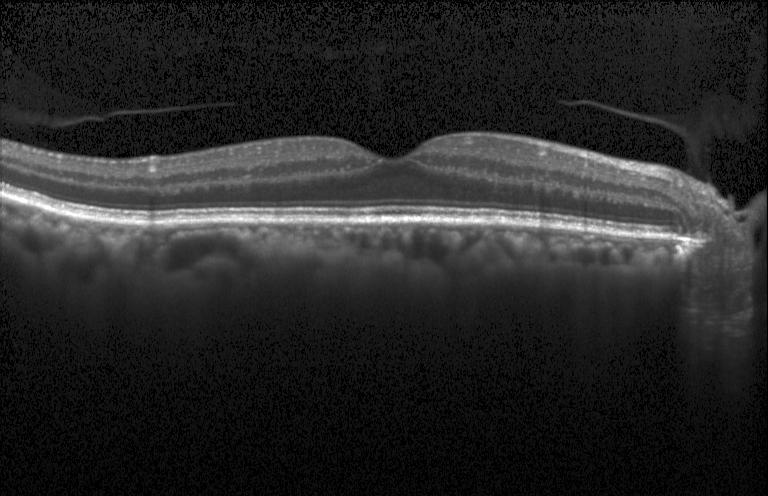 OCT scan showing no choroidal neovascularization, diabetic macular edema, or drusen.